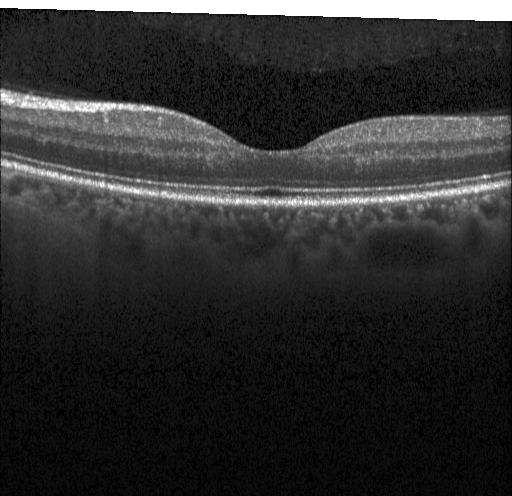
Macular OCT: neither choroidal neovascularization, diabetic macular edema, nor drusen.